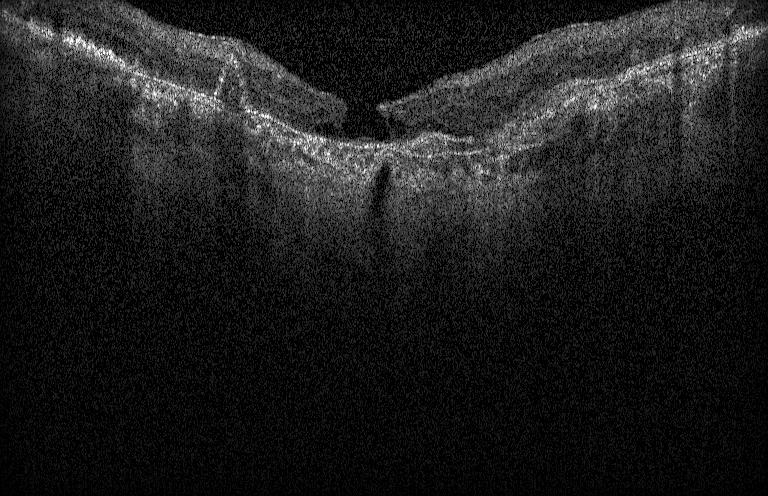
Optical coherence tomography B-scan.
A choroidal neovascular membrane.